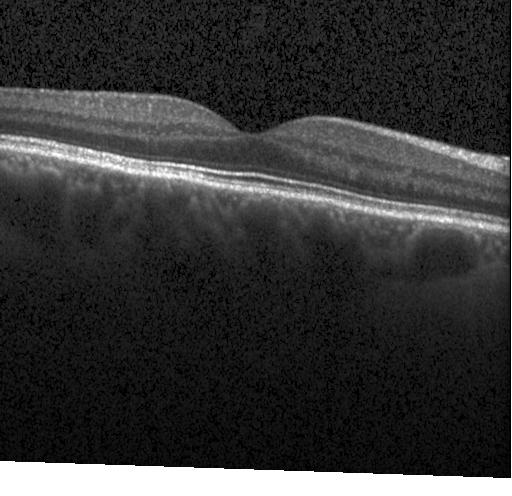
Spectral-domain OCT · through the macula · retinal OCT B-scan · instrument: Heidelberg Spectralis. Finding: no choroidal neovascularization, no diabetic macular edema, and no drusen.